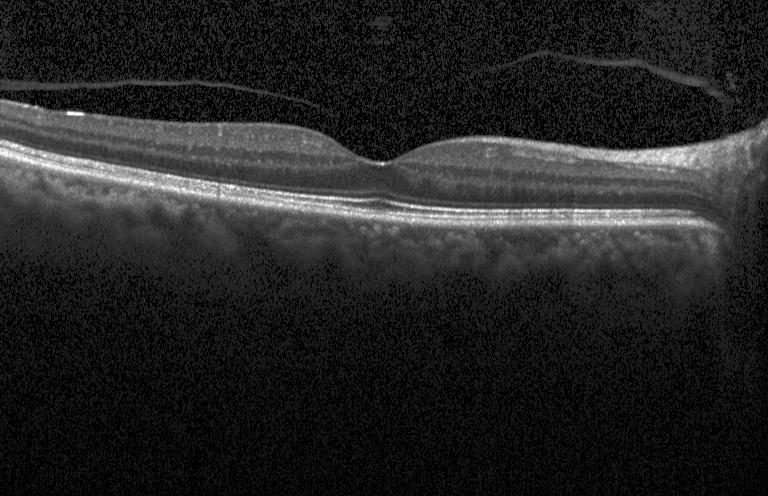 Optical coherence tomography scan. Macular OCT: no CNV, no DME, and no drusen.